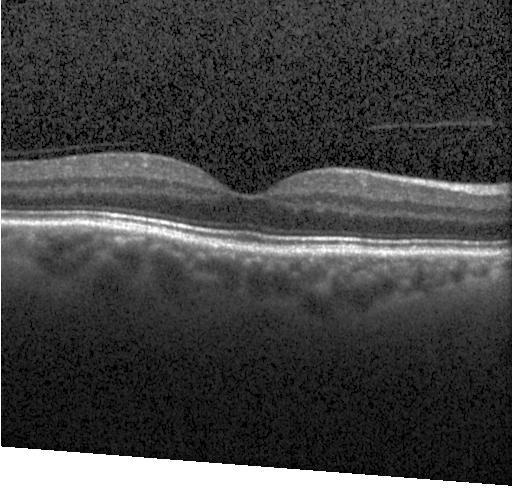
Optical coherence tomography scan.
Diagnosis: neither choroidal neovascularization, diabetic macular edema, nor drusen.